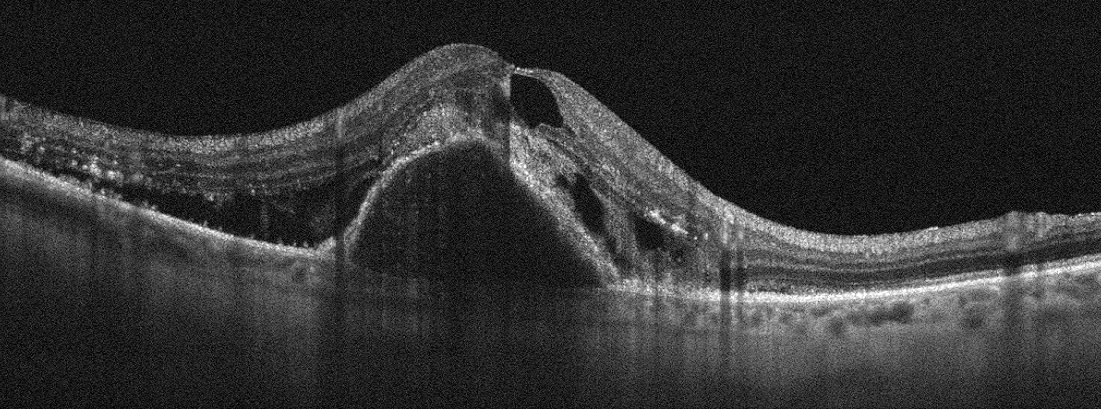

Through the macula. Optovue Avanti RTVue XR. Retinal OCT cross-section. Dx: age-related macular degeneration.